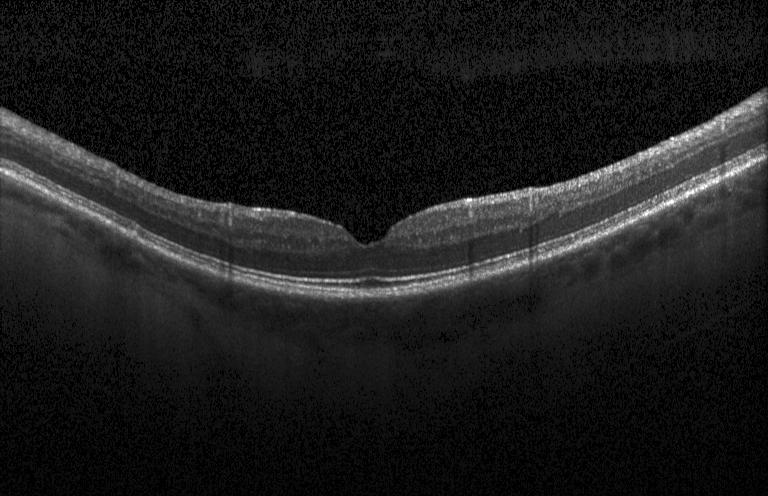
Retinal OCT cross-section. Diagnosis: no choroidal neovascularization, diabetic macular edema, or drusen.